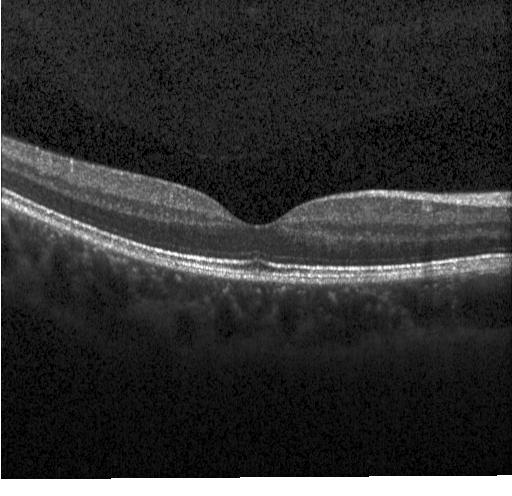
OCT B-scan · horizontal scan through the fovea.
No choroidal neovascularization, no diabetic macular edema, and no drusen.